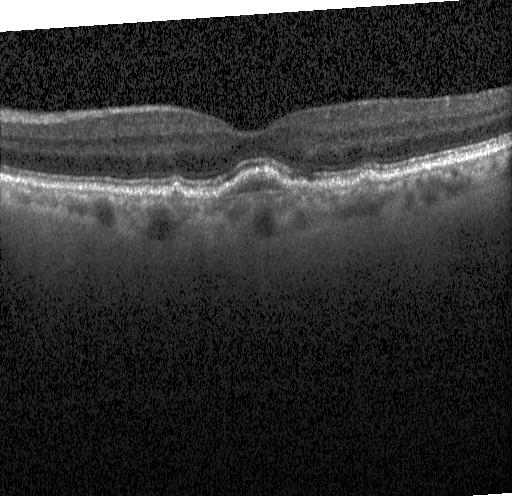
Optical coherence tomography scan · SD-OCT · instrument: Heidelberg Spectralis. Finding: a choroidal neovascular membrane.